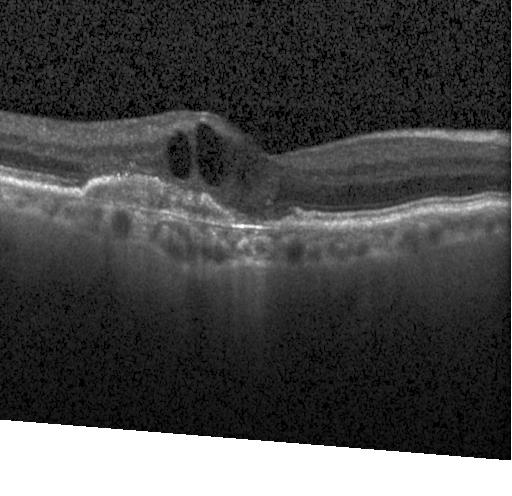 Retinal OCT cross-section — CNV.